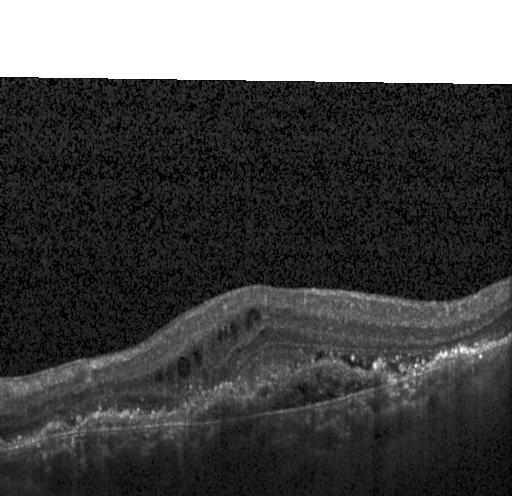
Macular scan, spectral-domain OCT, OCT line scan. Dx: CNV.